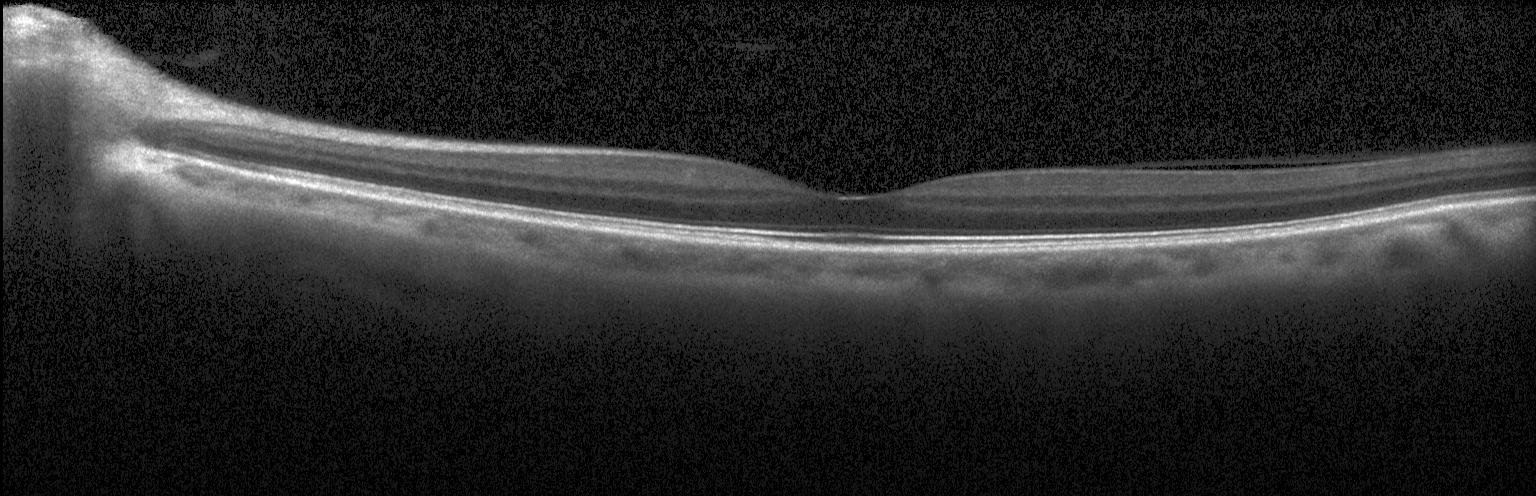 Optical coherence tomography scan · Heidelberg Spectralis · SD-OCT · macular scan. Dx: no choroidal neovascularization, no diabetic macular edema, and no drusen.